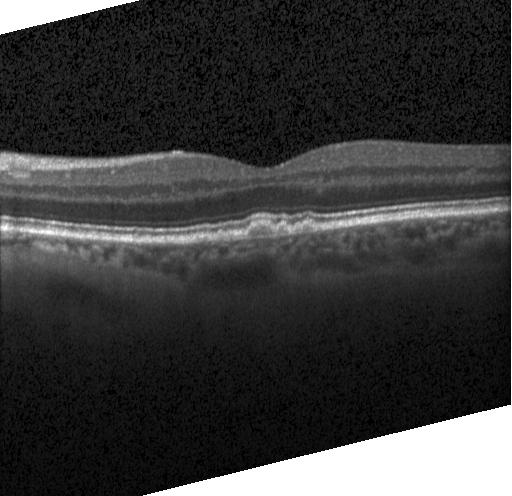

OCT B-scan; acquired on a Heidelberg Spectralis. The scan shows drusen.